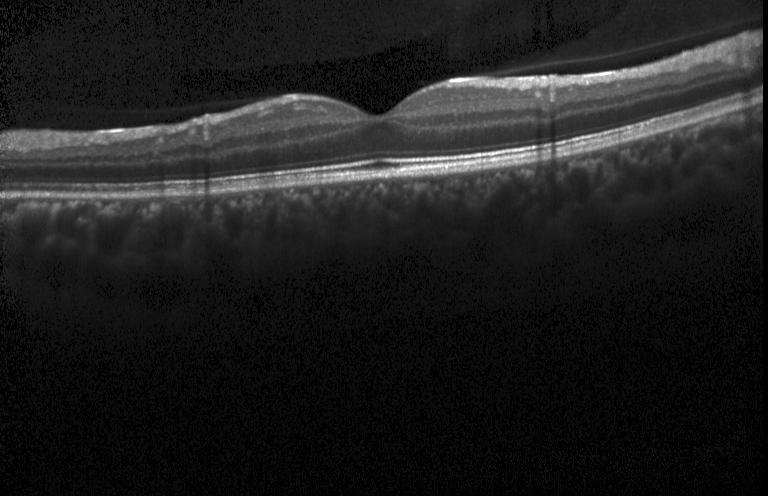

Diagnosis: no evidence of CNV, DME, or drusen.